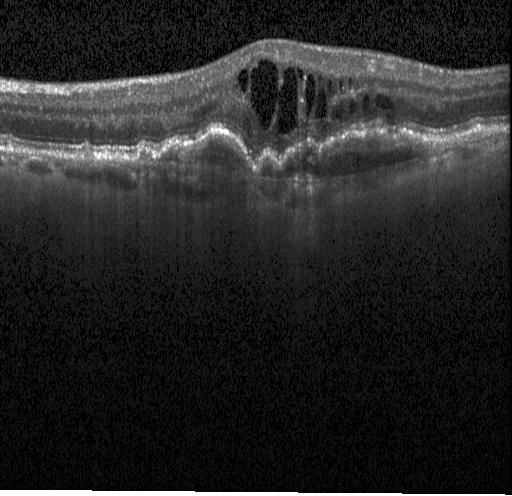 Centered on the fovea; OCT line scan; acquired on a Heidelberg Spectralis; SD-OCT — Macular OCT: a choroidal neovascular membrane.